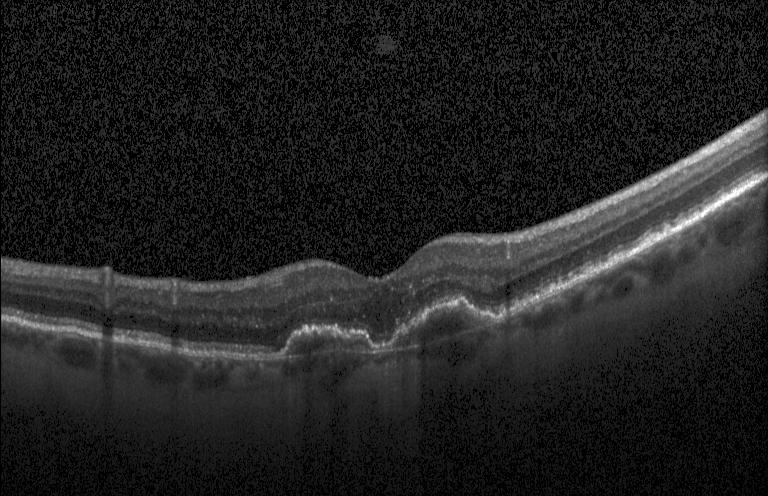

OCT B-scan; spectral-domain OCT — Impression: choroidal neovascularization (CNV).